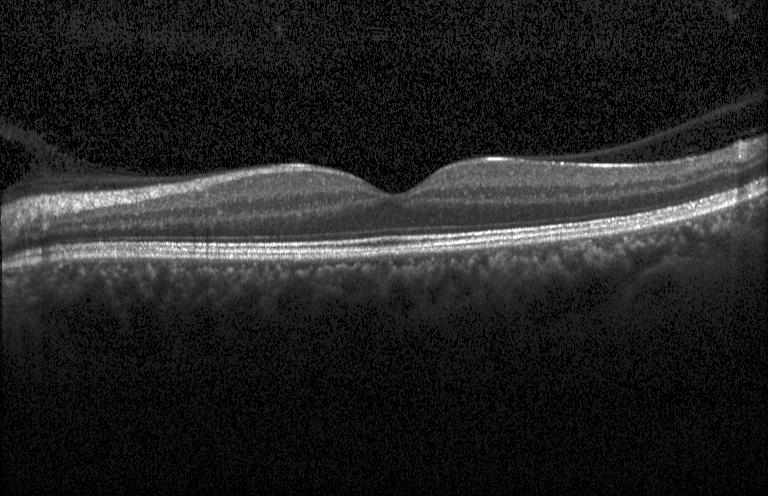
Heidelberg Spectralis OCT system, centered on the fovea, SD-OCT, retinal OCT B-scan — Assessment: neither choroidal neovascularization, diabetic macular edema, nor drusen.